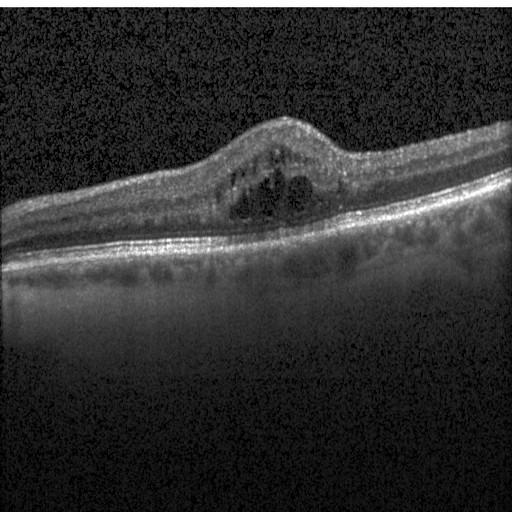 This B-scan demonstrates diabetic macular edema (DME).